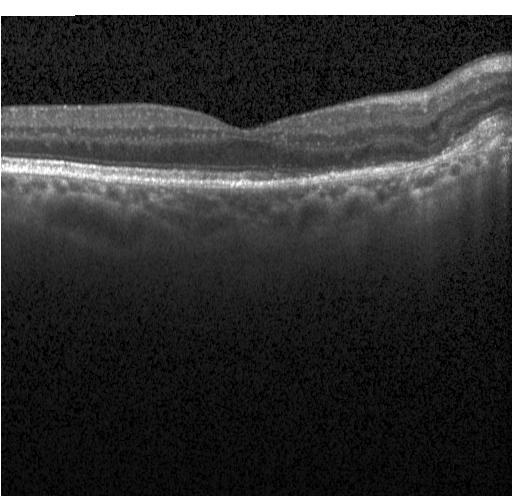
The scan shows choroidal neovascularization (CNV).